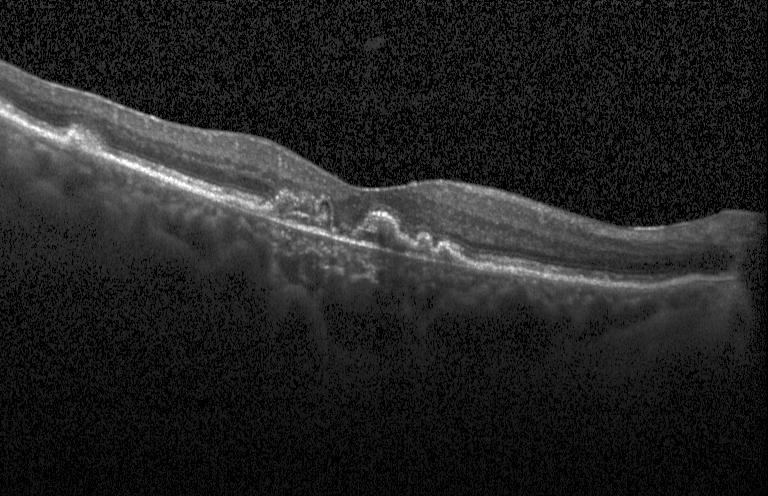
Spectral-domain optical coherence tomography · retinal OCT cross-section
Finding: choroidal neovascularization.